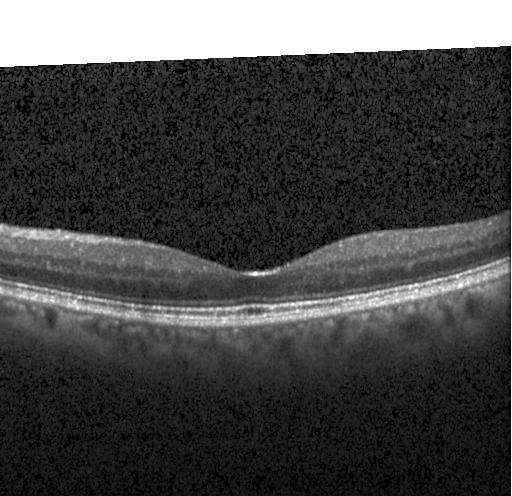

OCT B-scan. This B-scan demonstrates no CNV, no DME, and no drusen.